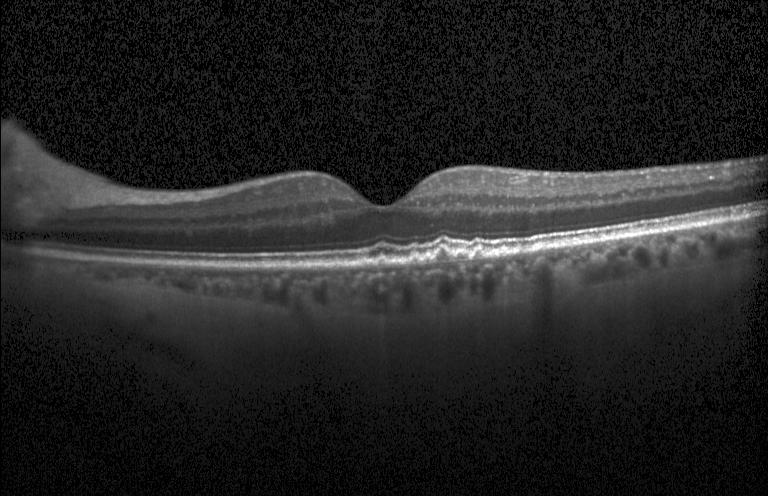

Retinal OCT cross-section · macular scan · spectral-domain optical coherence tomography
Finding: drusen.